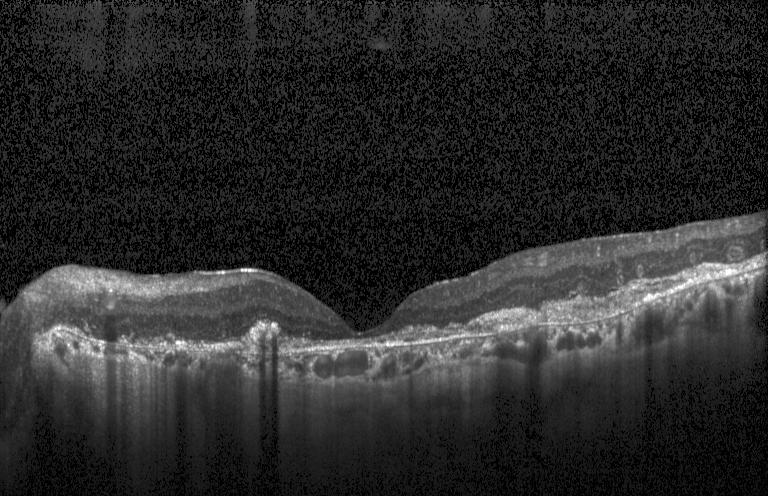
Spectral-domain optical coherence tomography · optical coherence tomography scan · Heidelberg Spectralis
Impression: a choroidal neovascular membrane.